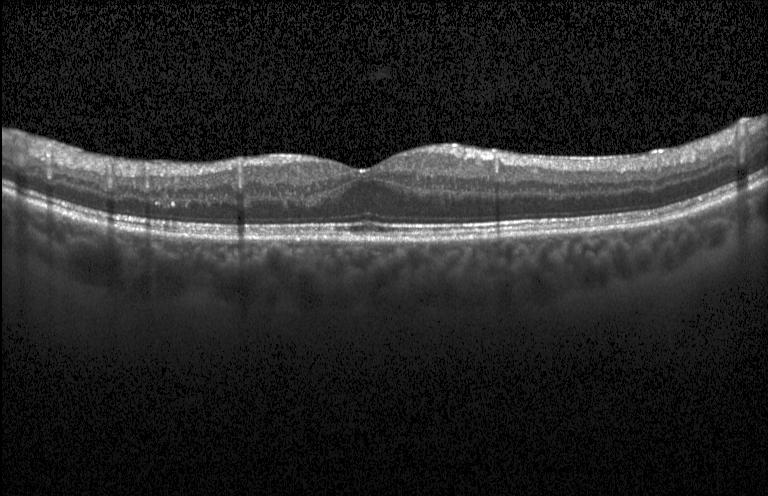

Retinal OCT B-scan; Heidelberg Spectralis OCT system.
Assessment: no choroidal neovascularization, diabetic macular edema, or drusen.